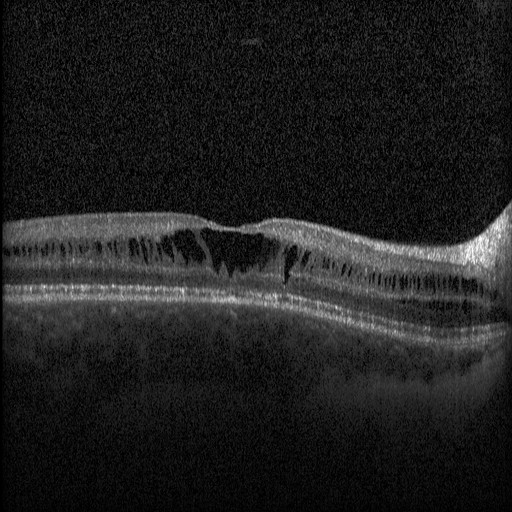
Optical coherence tomography scan; instrument: Heidelberg Spectralis. Dx: diabetic macular edema (DME).